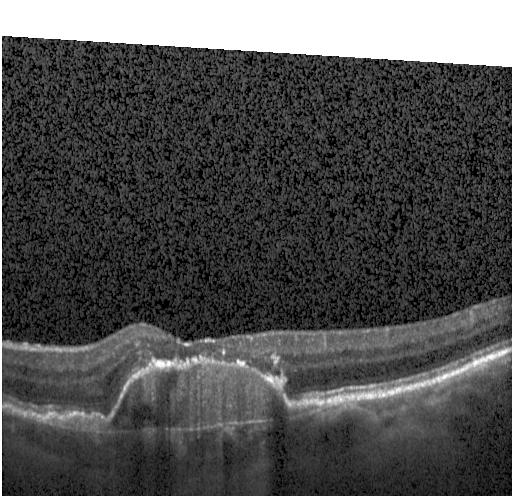 Impression: CNV.